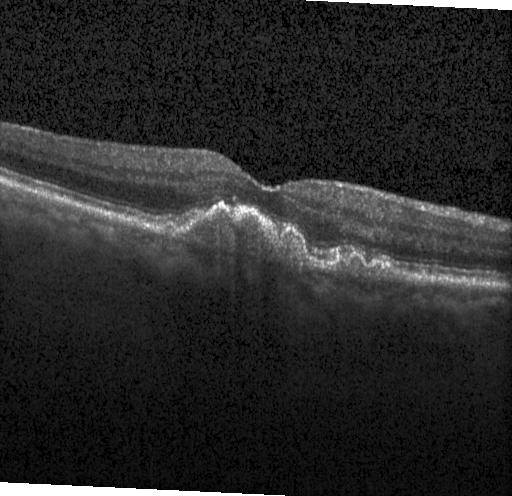 OCT B-scan, acquired on a Heidelberg Spectralis, SD-OCT
Diagnosis: a choroidal neovascular membrane.